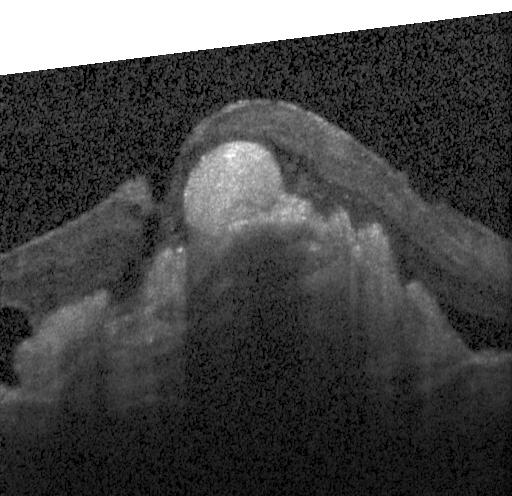
OCT scan showing a choroidal neovascular membrane.